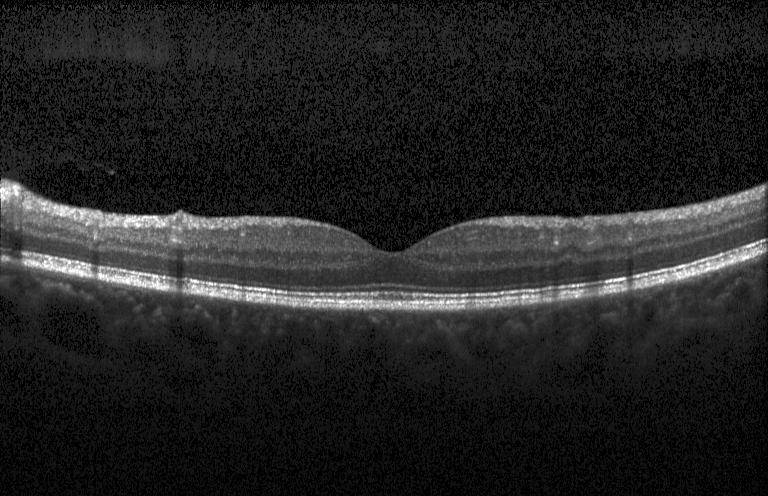
The scan shows no CNV, no DME, and no drusen.